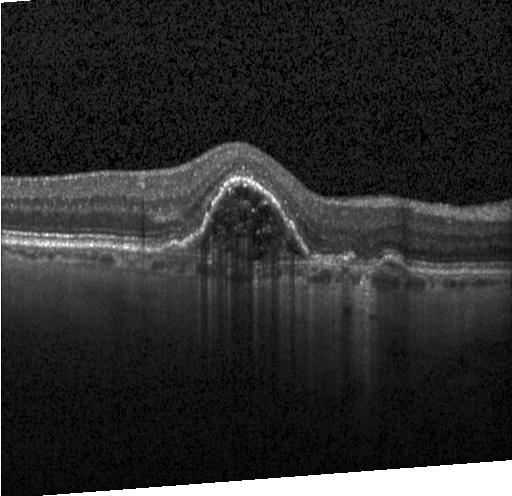

Instrument: Heidelberg Spectralis; spectral-domain optical coherence tomography; retinal OCT B-scan; centered on the fovea.
A choroidal neovascular membrane.